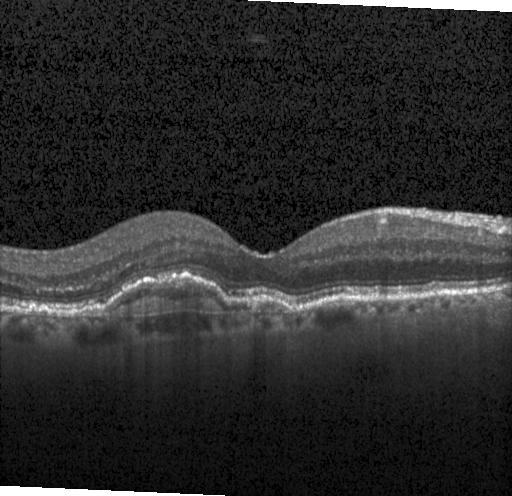

Retinal OCT B-scan. Spectral-domain OCT. Heidelberg Spectralis. Fovea-centered
The scan shows choroidal neovascularization (CNV).